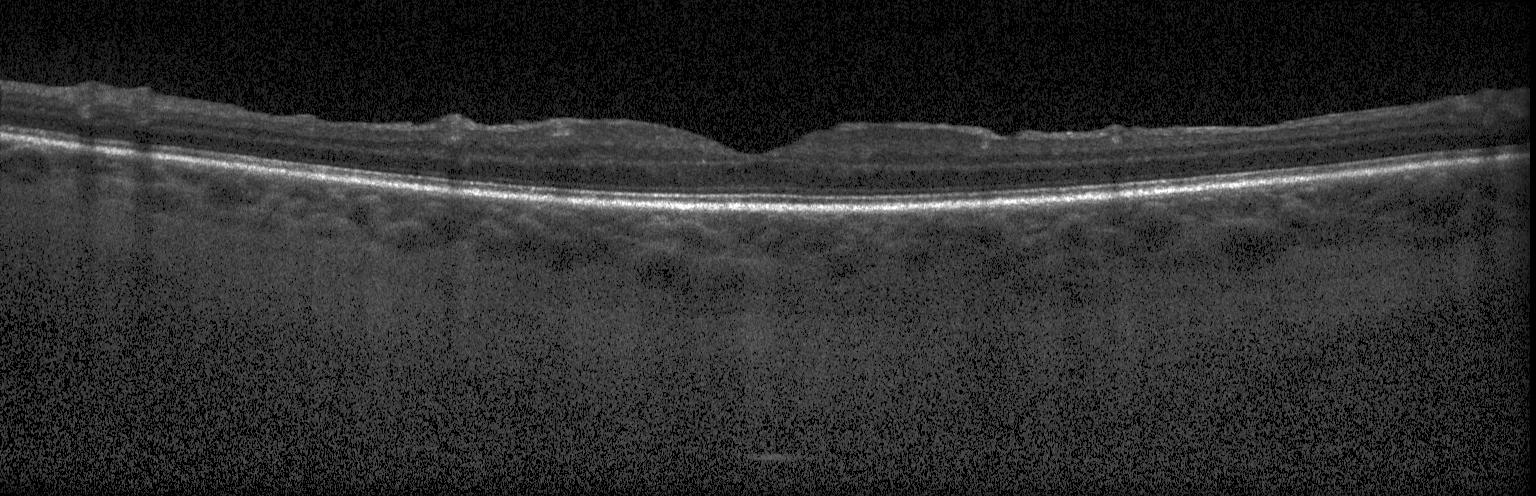
OCT scan showing no CNV, no DME, and no drusen.